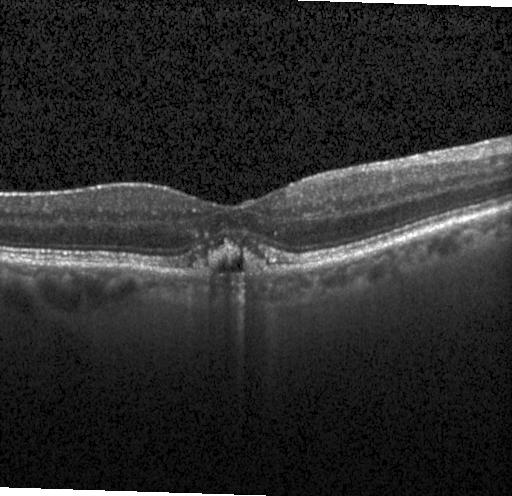
Retinal OCT cross-section; spectral-domain OCT
Impression: a choroidal neovascular membrane.